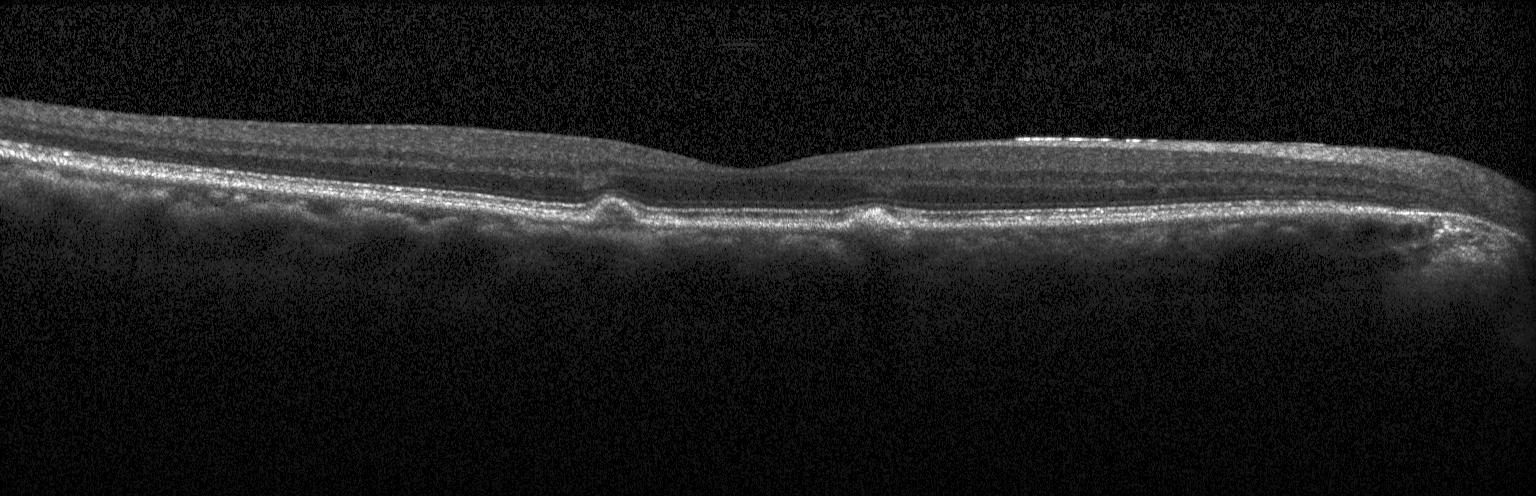 Dx: sub-RPE drusenoid deposits.